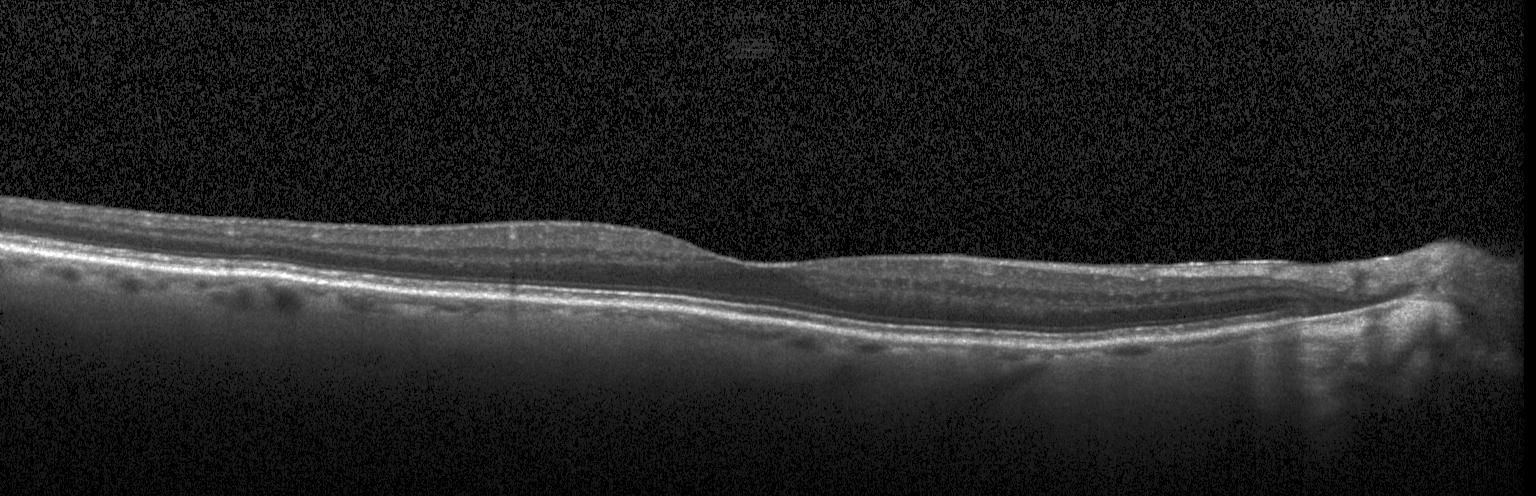

OCT line scan, spectral-domain OCT, Heidelberg Spectralis OCT system.
Finding: no evidence of choroidal neovascularization, diabetic macular edema, or drusen.